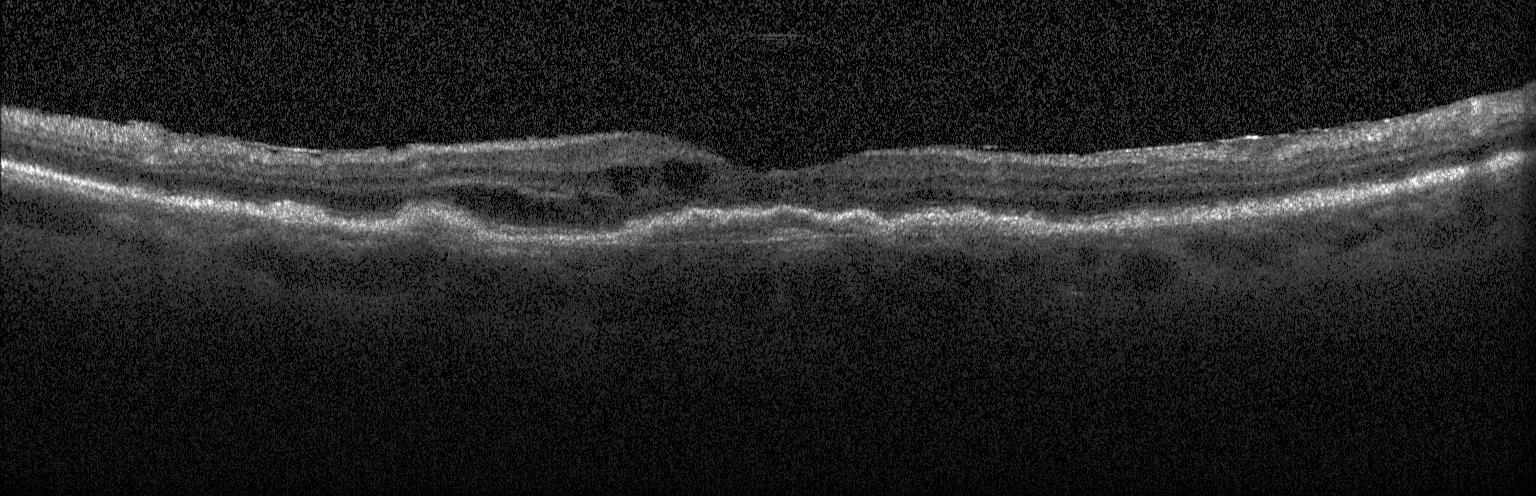

The scan shows a choroidal neovascular membrane.